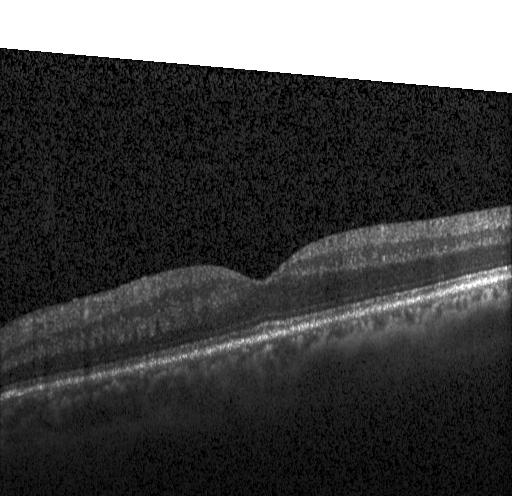 Spectral-domain optical coherence tomography, OCT B-scan.
Diagnosis: no evidence of choroidal neovascularization, diabetic macular edema, or drusen.